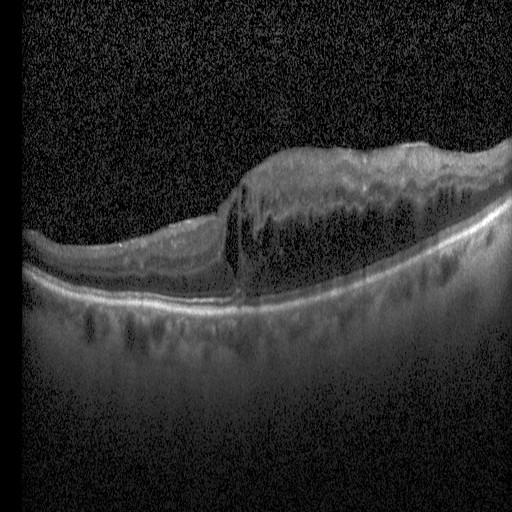

Spectral-domain OCT. OCT line scan. Acquired on a Heidelberg Spectralis. Centered on the fovea — OCT finding: diabetic macular edema.